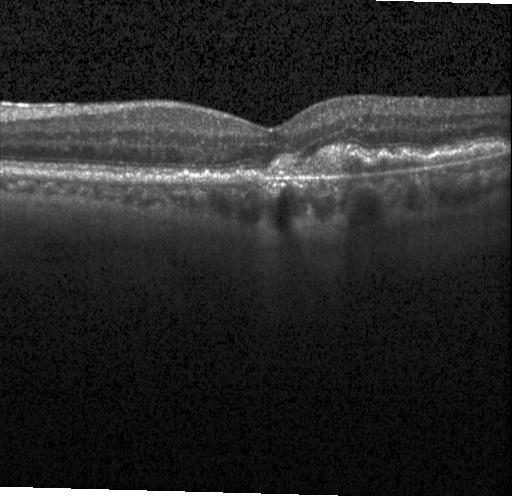 Optical coherence tomography B-scan. Spectral-domain OCT. Acquired on a Heidelberg Spectralis. Centered on the fovea. Finding: a choroidal neovascular membrane.